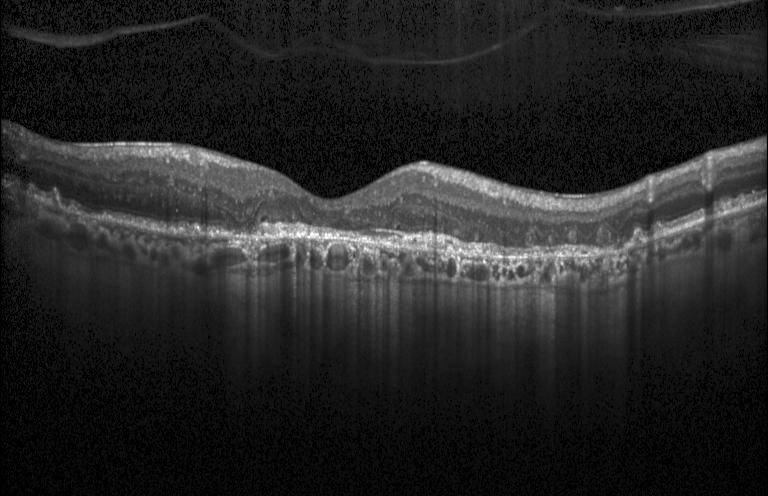 Instrument: Heidelberg Spectralis; spectral-domain optical coherence tomography; retinal OCT cross-section. OCT finding: choroidal neovascularization (CNV).